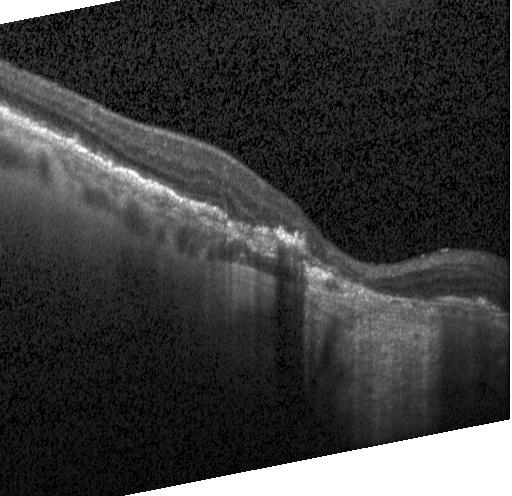 Spectral-domain OCT · retinal OCT cross-section · Heidelberg Spectralis · macular scan
Diagnosis: choroidal neovascularization (CNV).